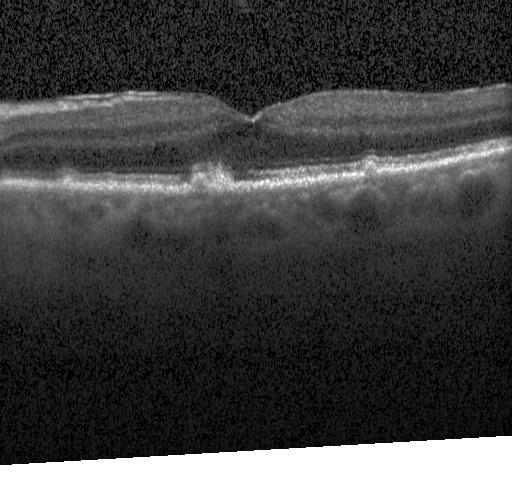
Optical coherence tomography B-scan. Heidelberg Spectralis OCT system
Impression: sub-RPE drusenoid deposits.